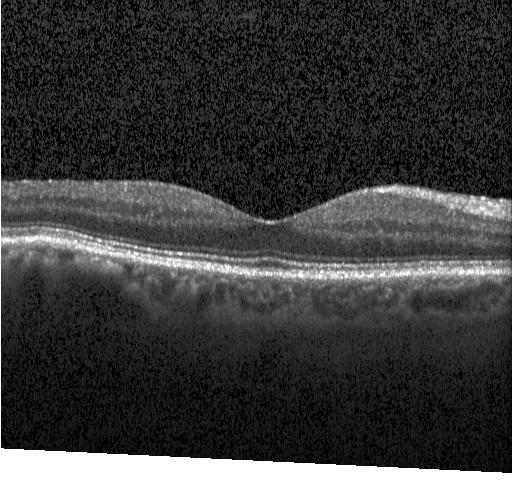 Spectral-domain OCT; optical coherence tomography scan; Heidelberg Spectralis OCT system; fovea-centered. Finding: neither choroidal neovascularization, diabetic macular edema, nor drusen.